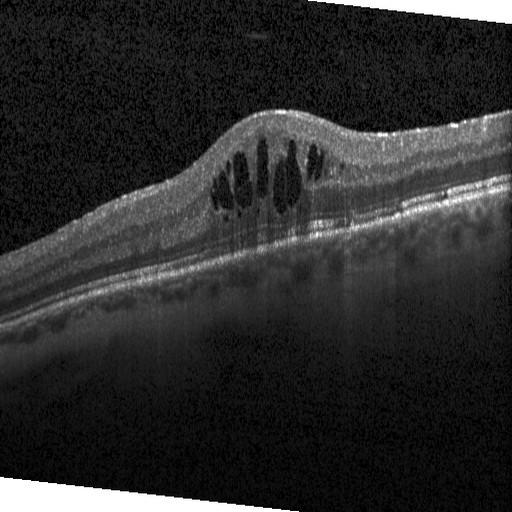 Macular OCT: diabetic macular edema.